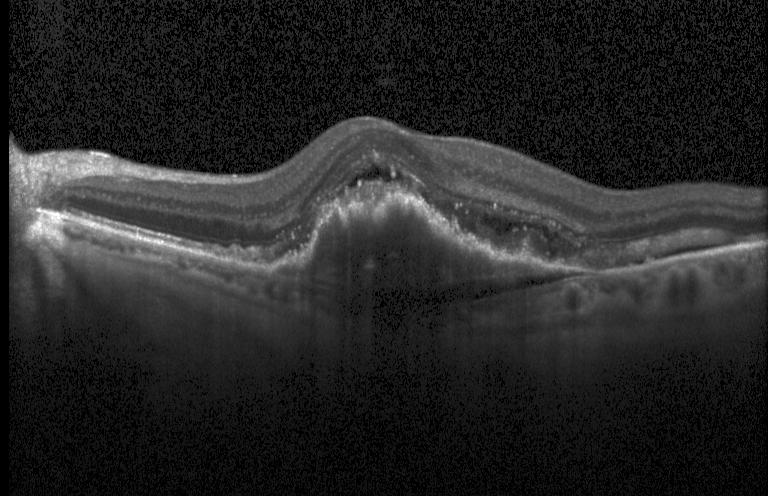 Macular OCT demonstrating a choroidal neovascular membrane.